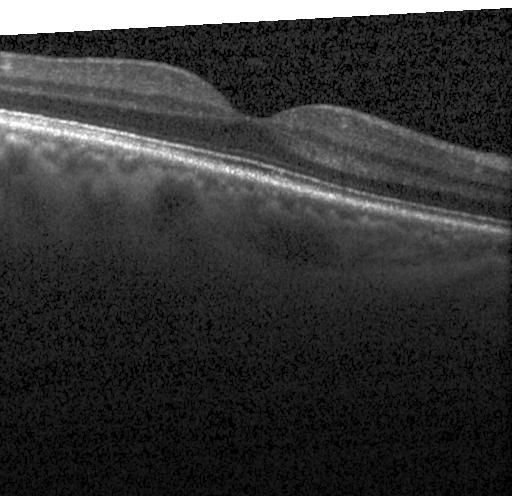
Retinal OCT B-scan; spectral-domain optical coherence tomography. Assessment: neither choroidal neovascularization, diabetic macular edema, nor drusen.